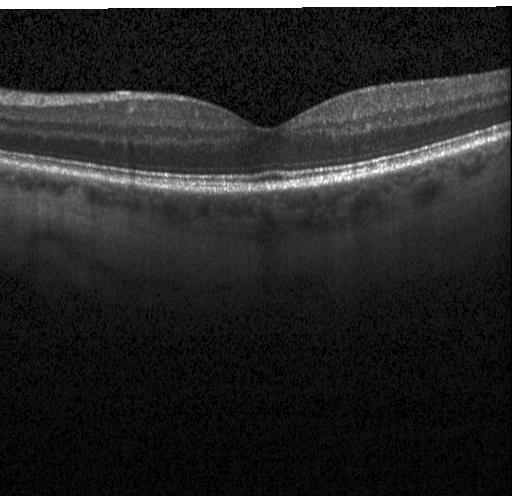
Finding: no choroidal neovascularization, no diabetic macular edema, and no drusen.